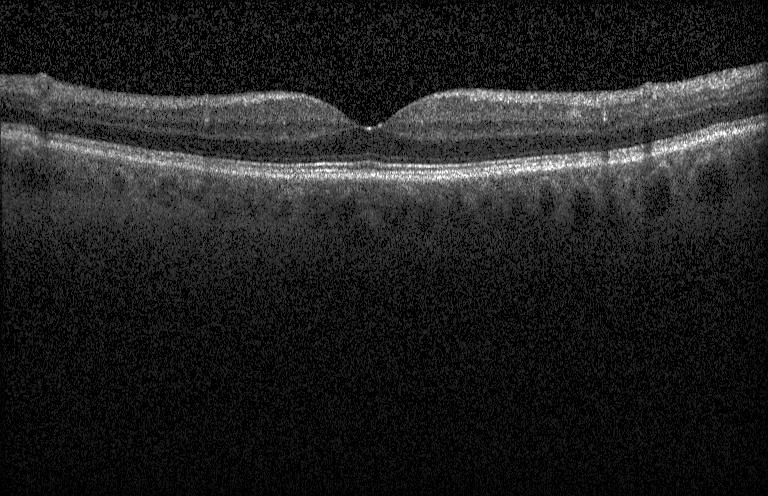 Heidelberg Spectralis, spectral-domain OCT, macular scan, OCT B-scan — Dx: no evidence of CNV, DME, or drusen.